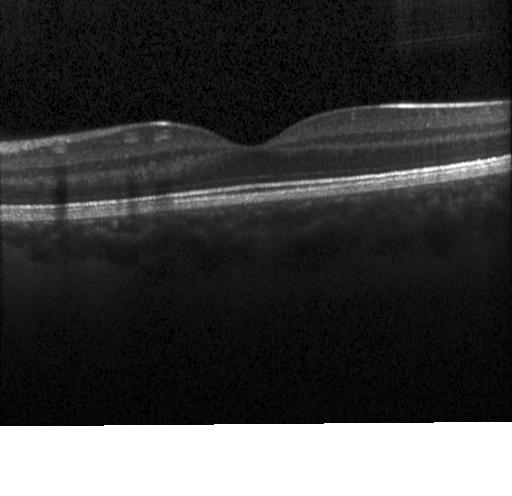
Retinal OCT cross-section showing neither choroidal neovascularization, diabetic macular edema, nor drusen.